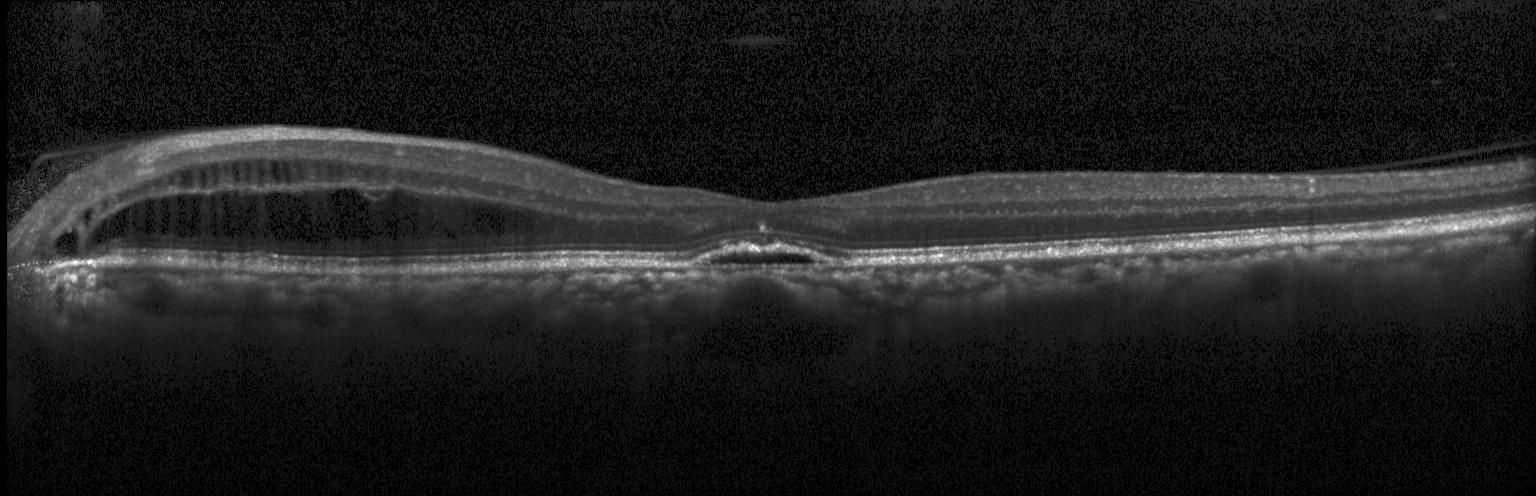

Fovea-centered; OCT line scan — Impression: CNV.